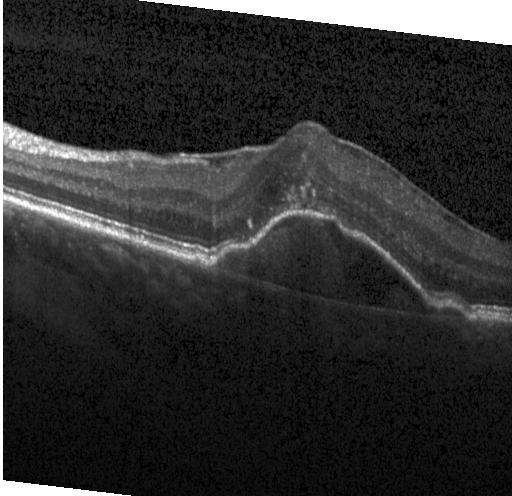

Heidelberg Spectralis; optical coherence tomography B-scan; spectral-domain optical coherence tomography. Diagnosis: a choroidal neovascular membrane.